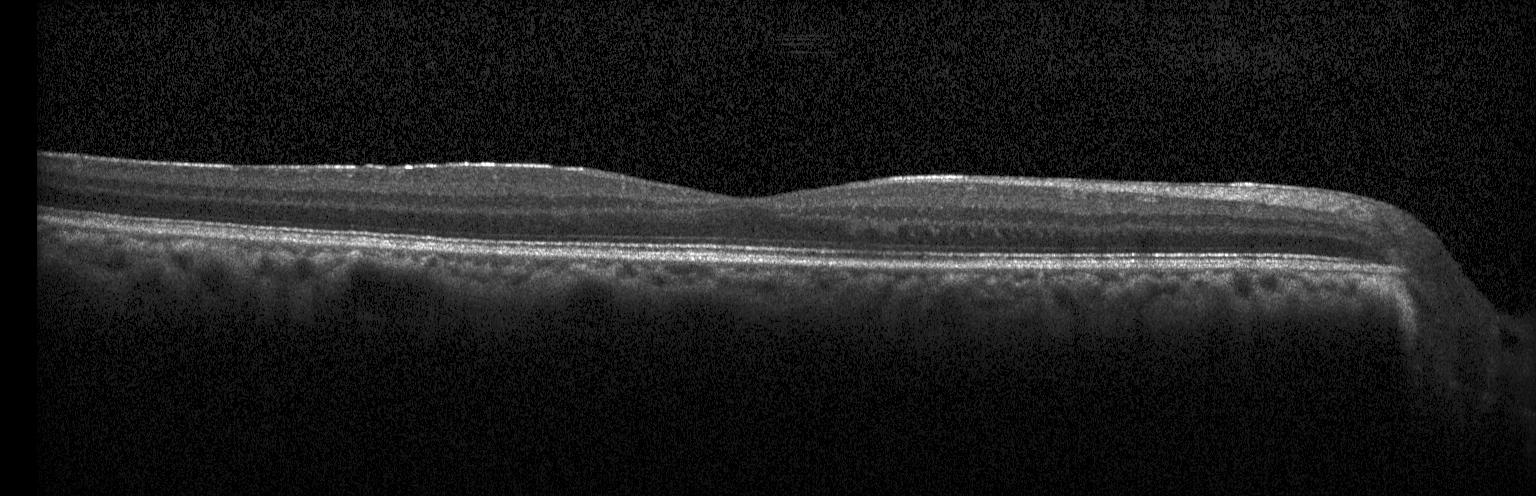 Optical coherence tomography B-scan.
Finding: neither CNV, DME, nor drusen.